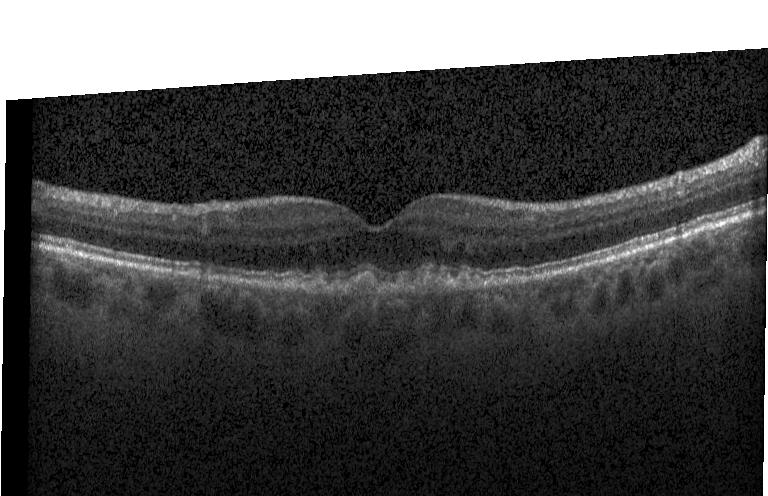
OCT B-scan showing multiple drusen.